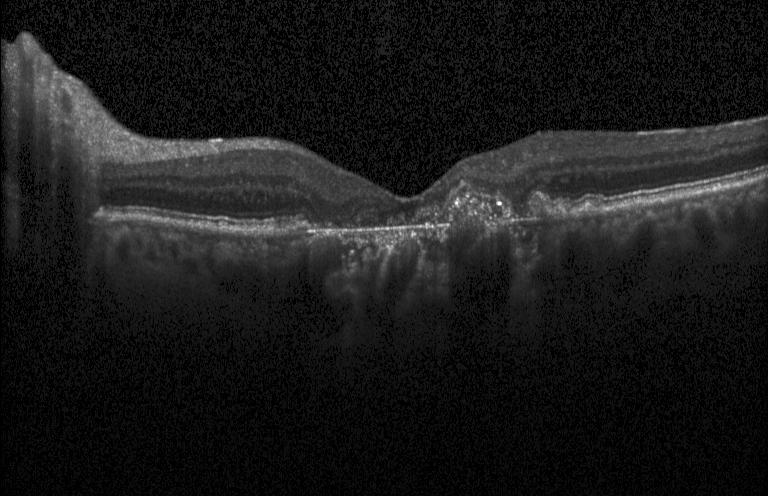

OCT finding: a choroidal neovascular membrane.